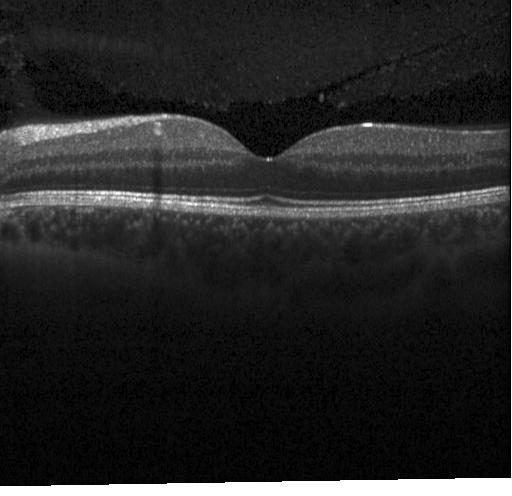

OCT finding: no choroidal neovascularization, diabetic macular edema, or drusen.